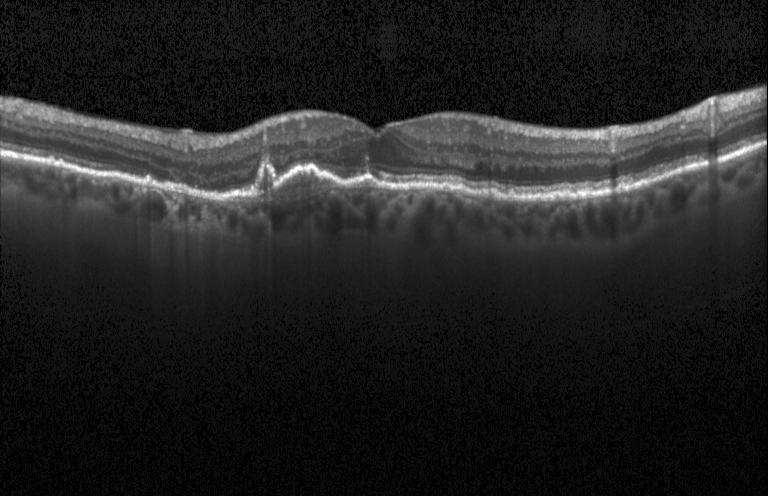 Retinal OCT B-scan, Heidelberg Spectralis OCT system, horizontal scan through the fovea. Finding: a choroidal neovascular membrane.